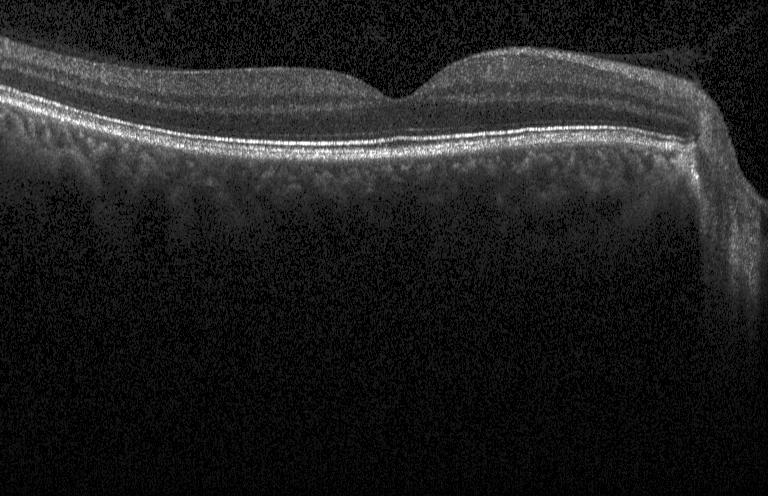 Spectral-domain OCT, OCT line scan, through the macula, acquired on a Heidelberg Spectralis — This B-scan demonstrates no choroidal neovascularization, no diabetic macular edema, and no drusen.